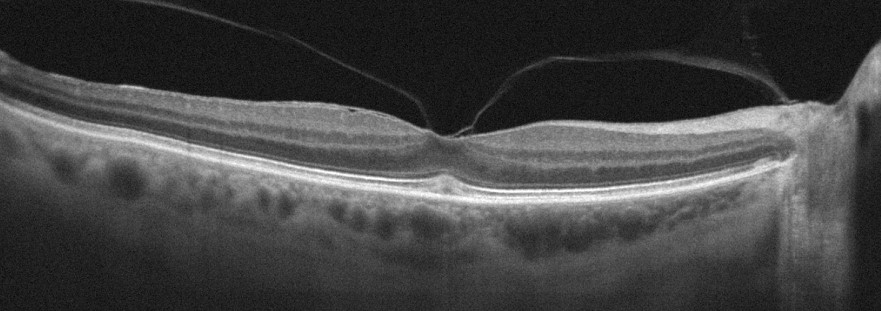

OCT B-scan — The scan shows vitreomacular interface disease (VID).